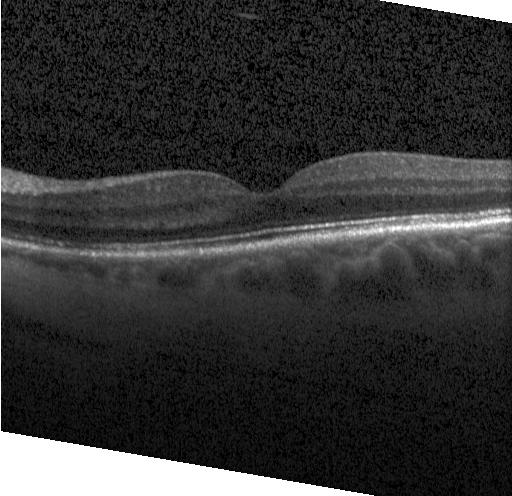

SD-OCT; optical coherence tomography B-scan.
This B-scan demonstrates no evidence of CNV, DME, or drusen.